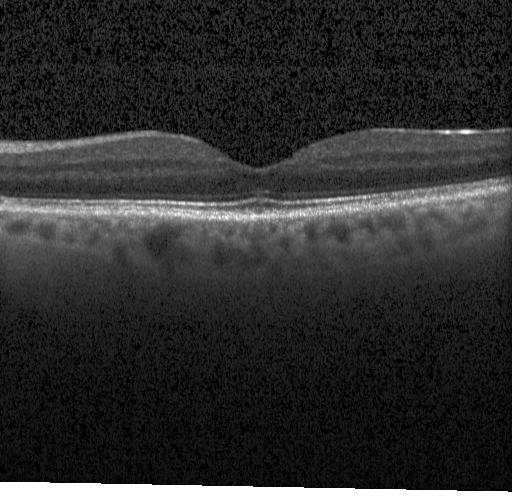
No choroidal neovascularization, diabetic macular edema, or drusen.